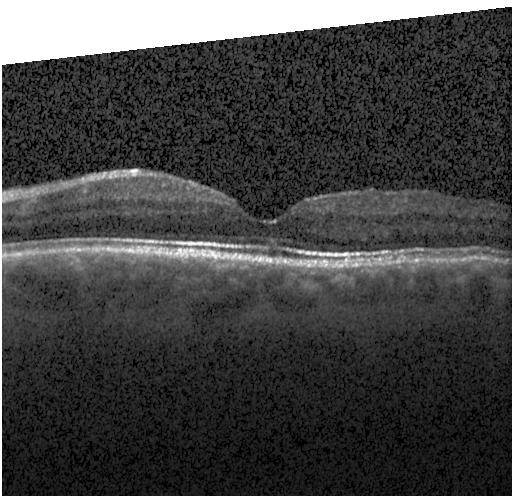 Diagnosis: no choroidal neovascularization, no diabetic macular edema, and no drusen.